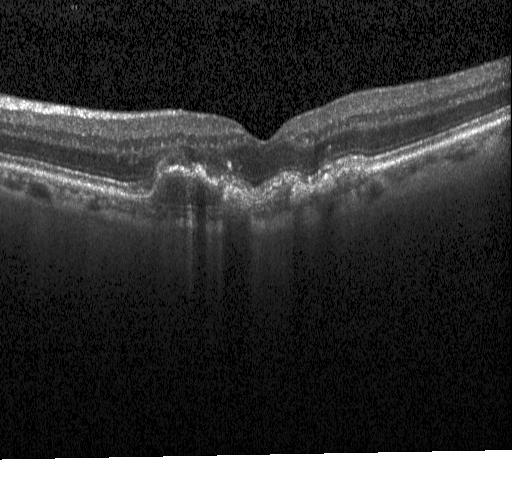

Finding: CNV.